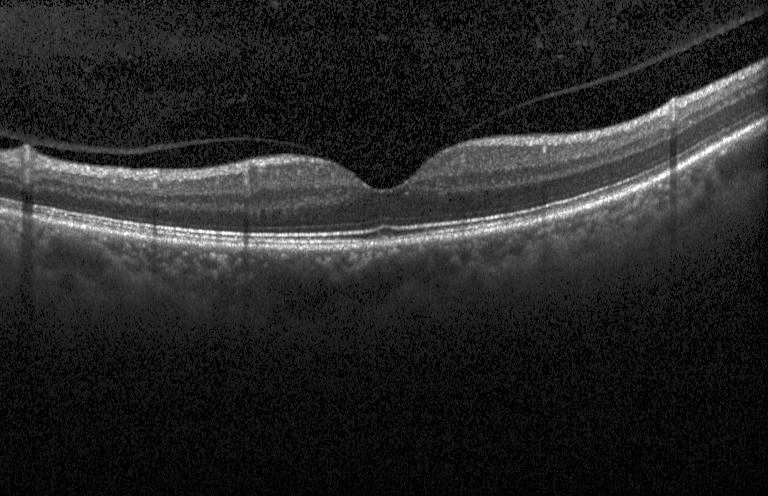

Heidelberg Spectralis OCT system. Retinal OCT B-scan. Diagnosis: no evidence of choroidal neovascularization, diabetic macular edema, or drusen.